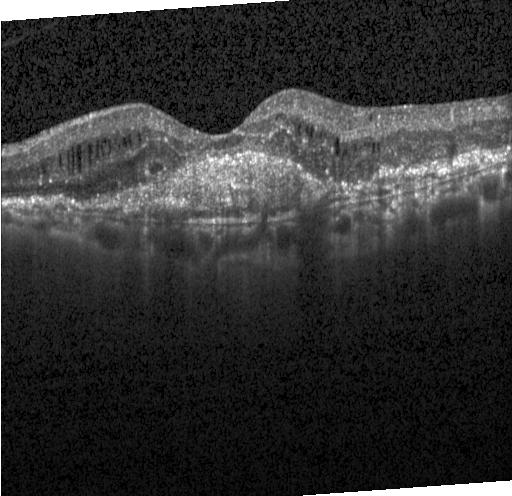
Retinal OCT B-scan, acquired on a Heidelberg Spectralis. Diagnosis: a choroidal neovascular membrane.